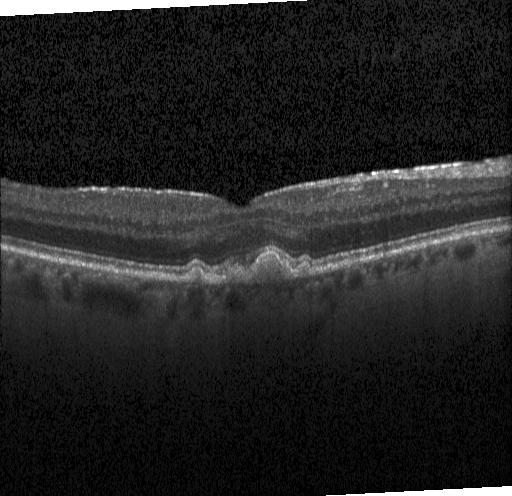 This B-scan demonstrates multiple drusen.